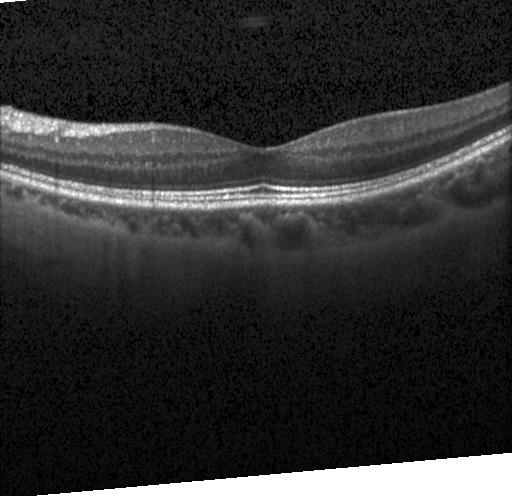
Diagnosis: no evidence of CNV, DME, or drusen.